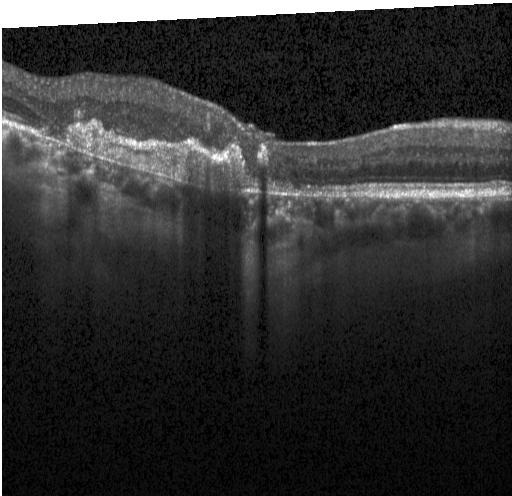

Retinal OCT cross-section. Heidelberg Spectralis OCT system
Diagnosis: CNV.